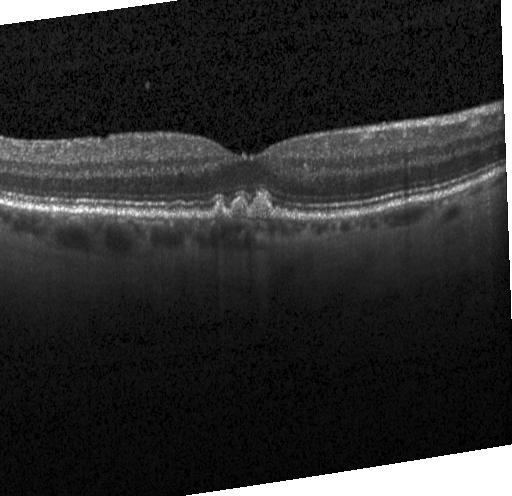 Impression: sub-RPE drusenoid deposits.